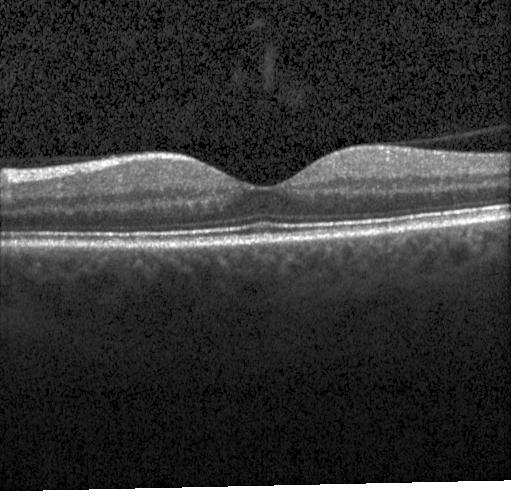

Fovea-centered; SD-OCT; optical coherence tomography scan
Macular OCT: no evidence of choroidal neovascularization, diabetic macular edema, or drusen.